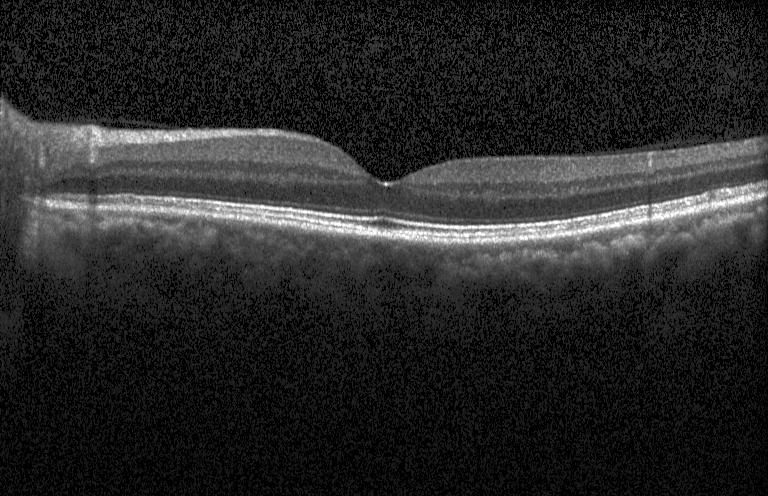

OCT line scan. Finding: no choroidal neovascularization, diabetic macular edema, or drusen.